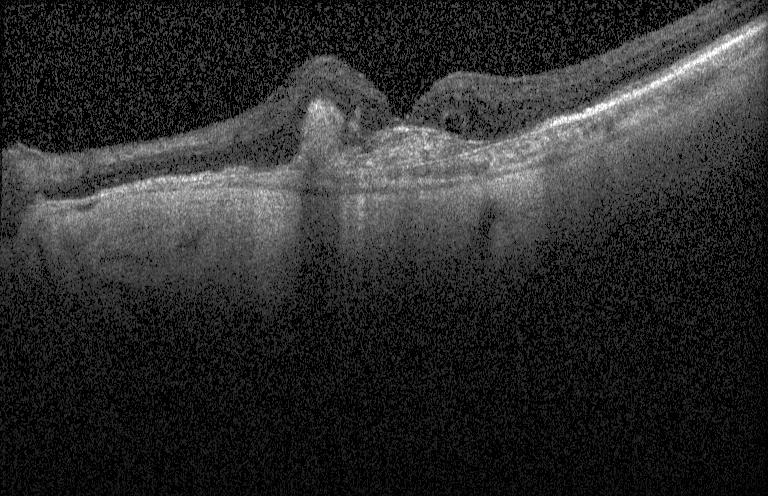
Dx: choroidal neovascularization.